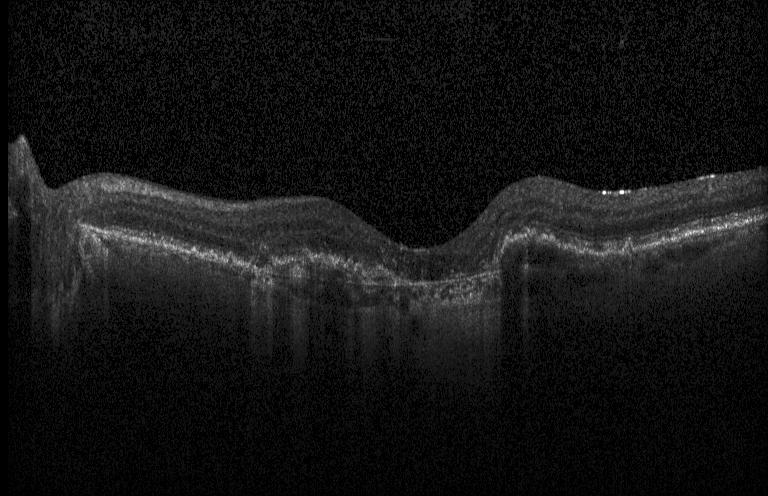
Retinal OCT cross-section showing choroidal neovascularization.